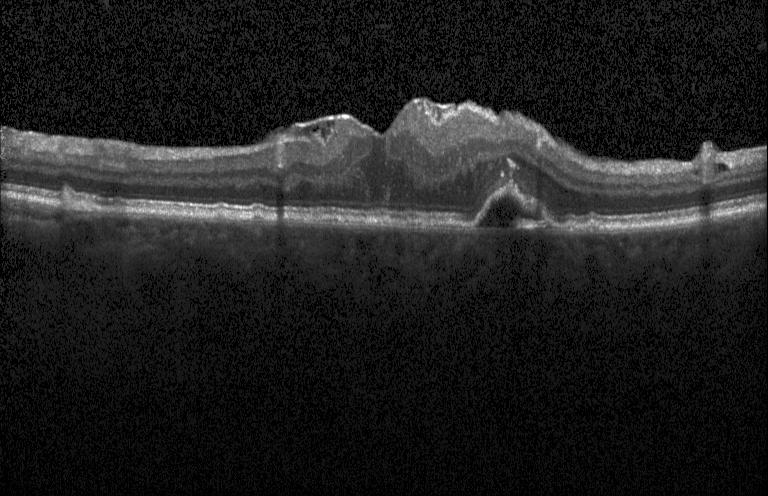

Impression: choroidal neovascularization.